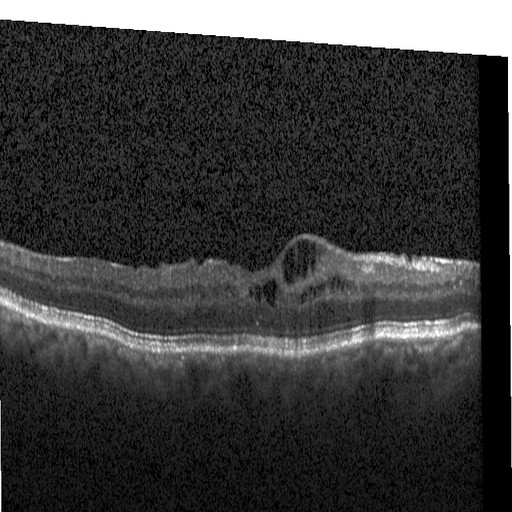 OCT line scan.
Diabetic macular edema (DME).